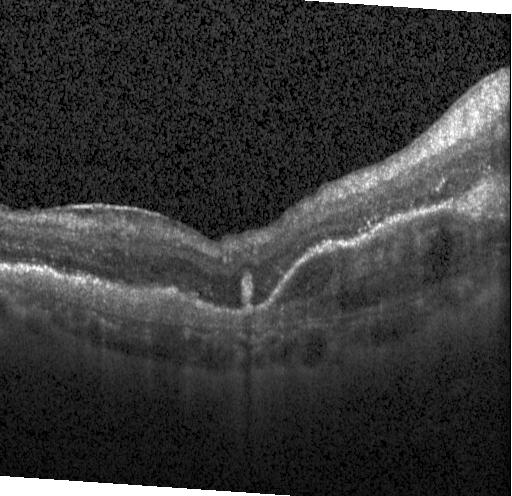
Optical coherence tomography scan.
The scan shows a choroidal neovascular membrane.